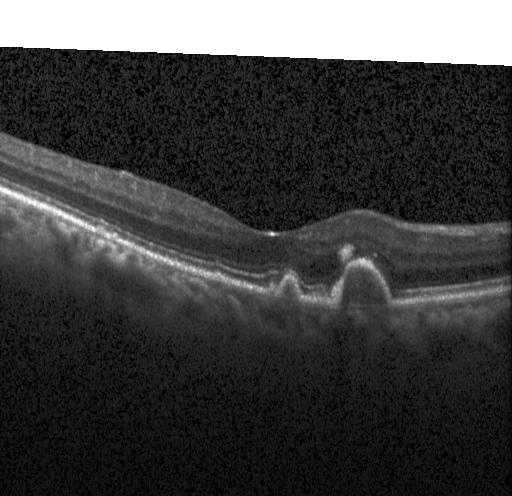

OCT line scan.
OCT finding: sub-RPE drusenoid deposits.